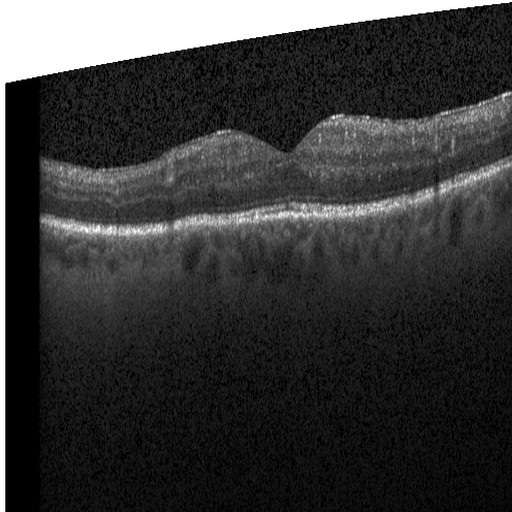
SD-OCT. Retinal OCT cross-section. Through the macula. Heidelberg Spectralis OCT system — Dx: diabetic macular edema (DME).